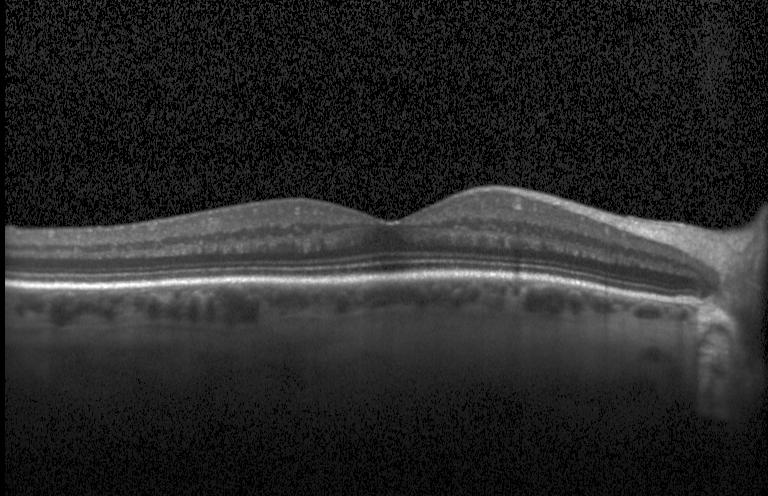

Macular OCT: neither choroidal neovascularization, diabetic macular edema, nor drusen.